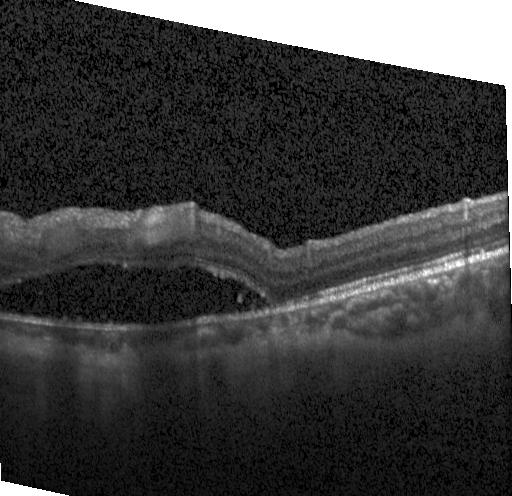 Finding: a choroidal neovascular membrane.